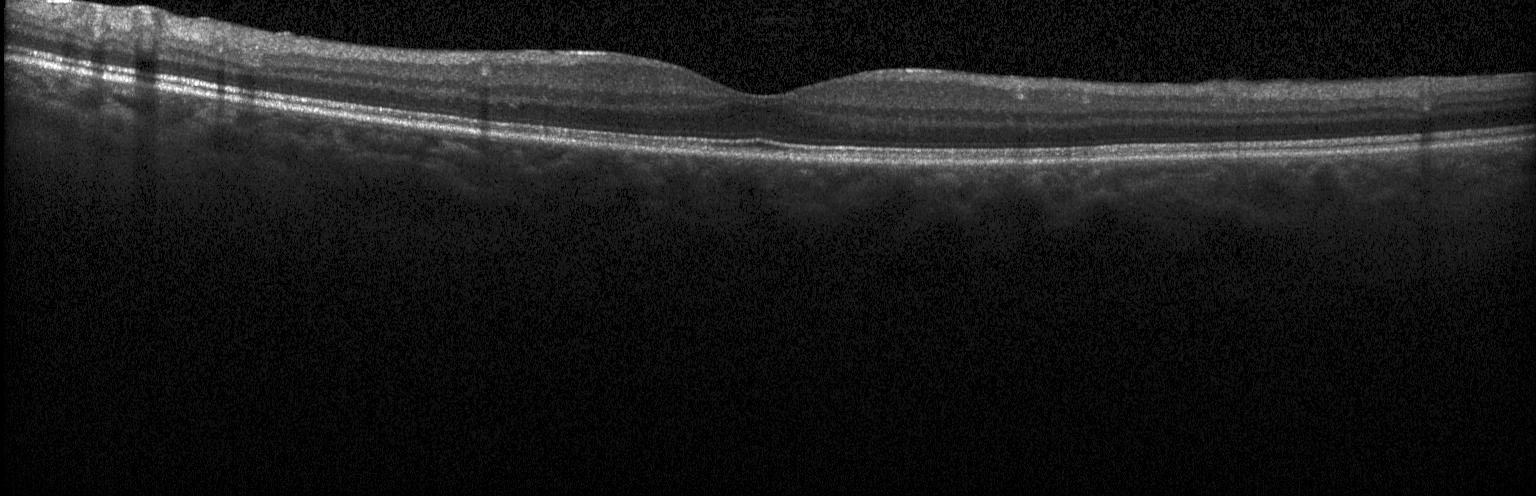 Dx: no choroidal neovascularization, diabetic macular edema, or drusen.